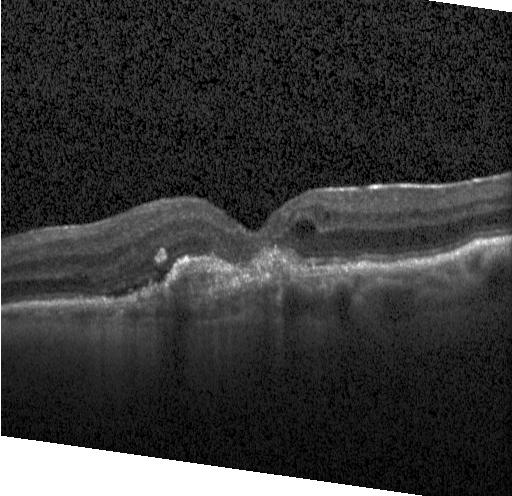
Finding: a choroidal neovascular membrane.